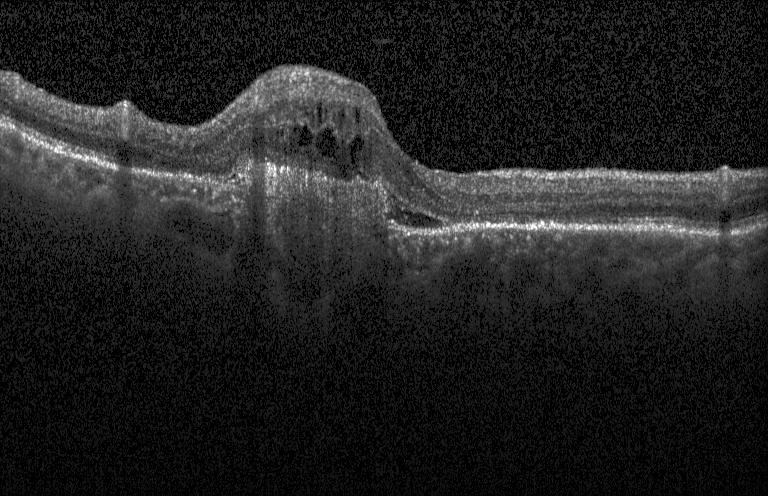

Macular scan. Spectral-domain OCT. OCT line scan. Finding: a choroidal neovascular membrane.